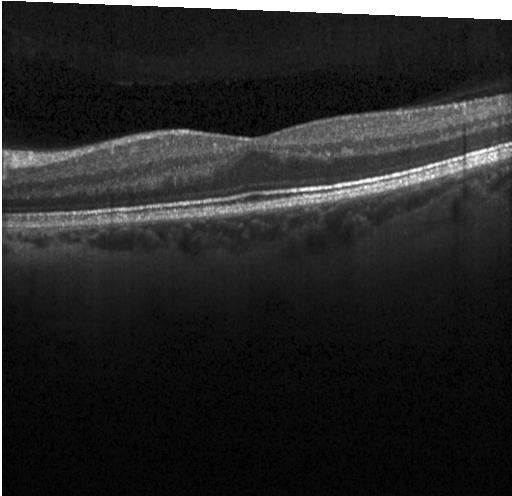 Heidelberg Spectralis OCT system · SD-OCT · optical coherence tomography B-scan.
Impression: neither choroidal neovascularization, diabetic macular edema, nor drusen.